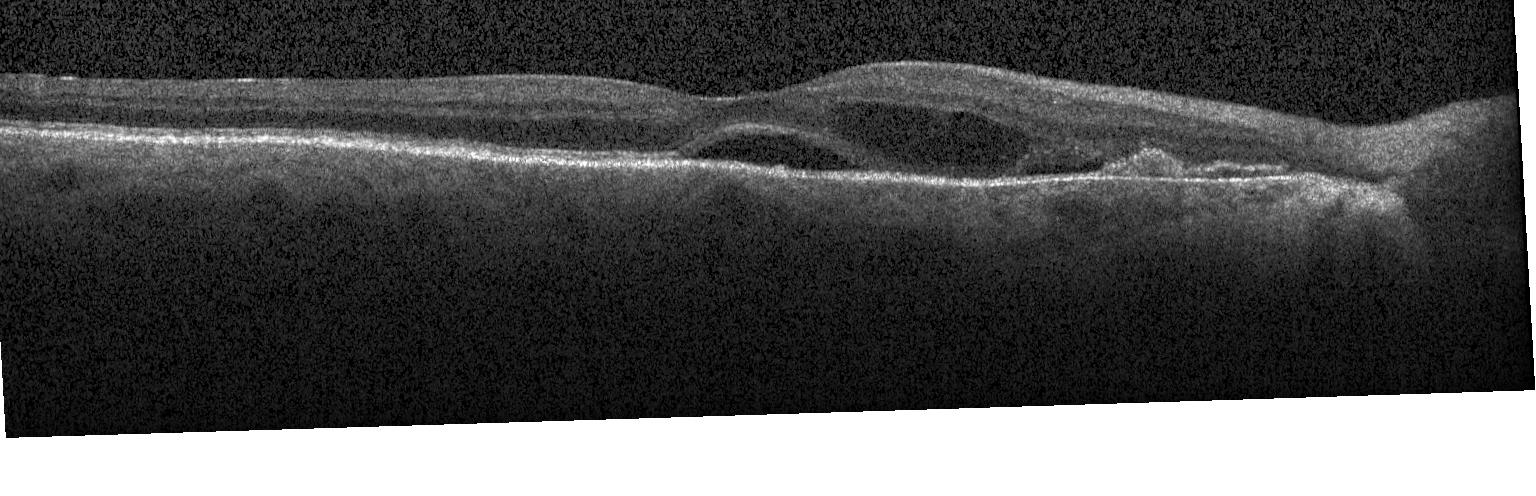
Instrument: Heidelberg Spectralis, OCT B-scan, spectral-domain optical coherence tomography. A choroidal neovascular membrane.